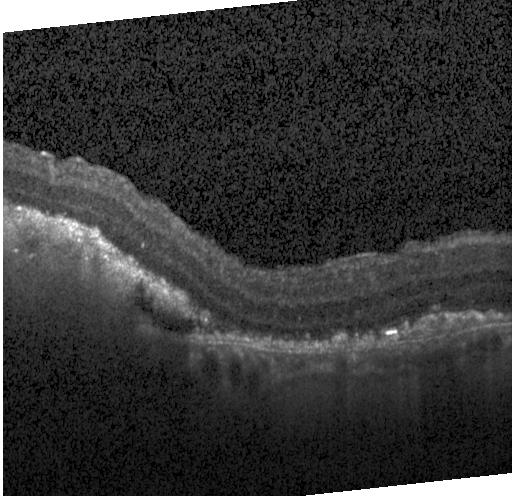
Spectral-domain OCT B-scan: a choroidal neovascular membrane.